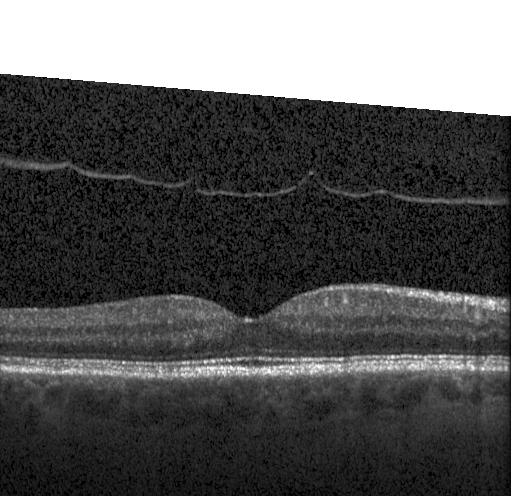

OCT line scan — This B-scan demonstrates no evidence of CNV, DME, or drusen.